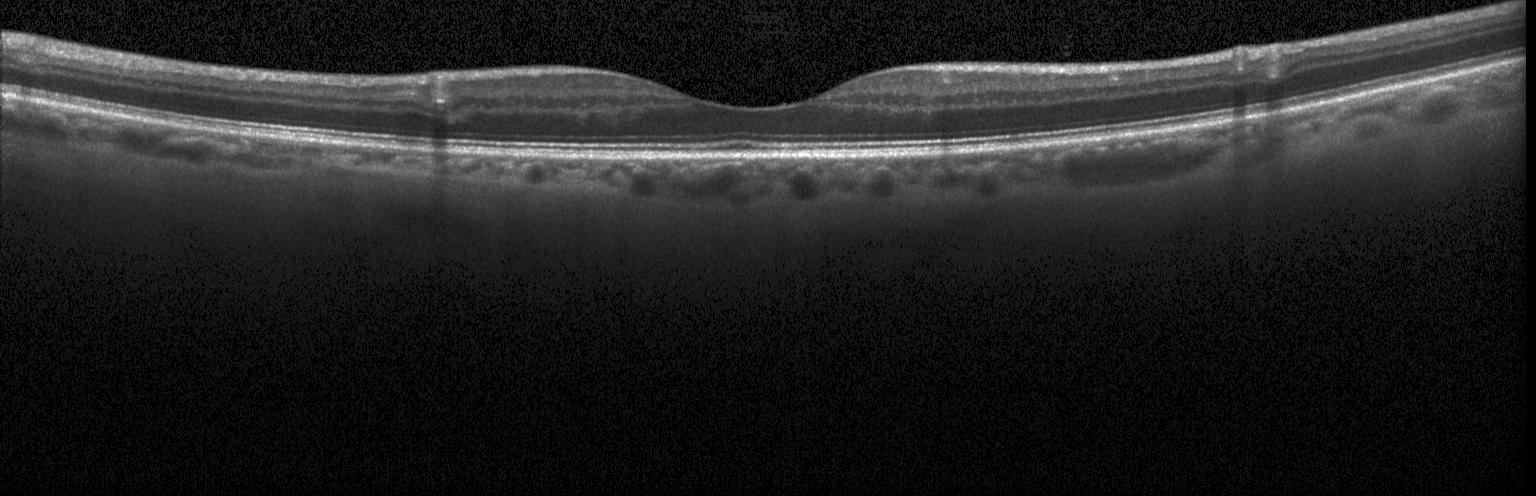 Instrument: Heidelberg Spectralis, SD-OCT, through the macula, OCT line scan — Finding: no evidence of CNV, DME, or drusen.